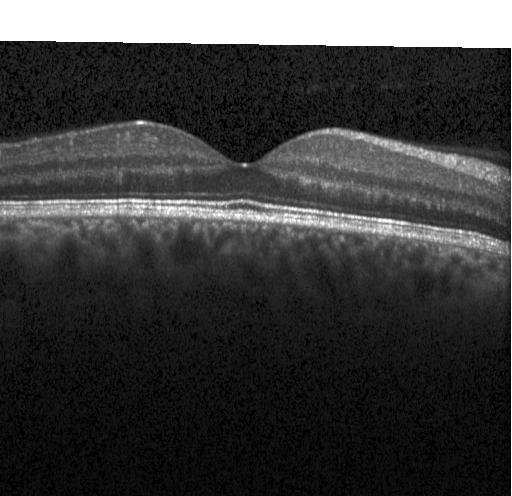

Optical coherence tomography scan — Macular OCT: no choroidal neovascularization, no diabetic macular edema, and no drusen.